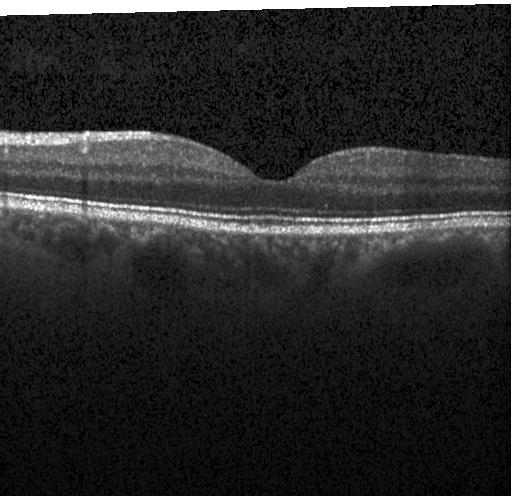 OCT B-scan. Finding: no choroidal neovascularization, no diabetic macular edema, and no drusen.